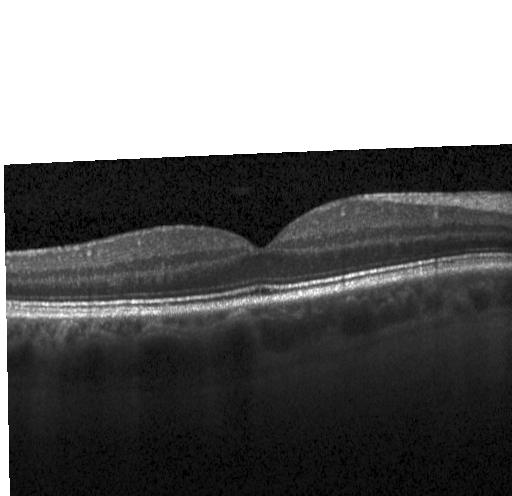 Spectral-domain optical coherence tomography, optical coherence tomography B-scan, Heidelberg Spectralis, macular scan
Diagnosis: no evidence of choroidal neovascularization, diabetic macular edema, or drusen.